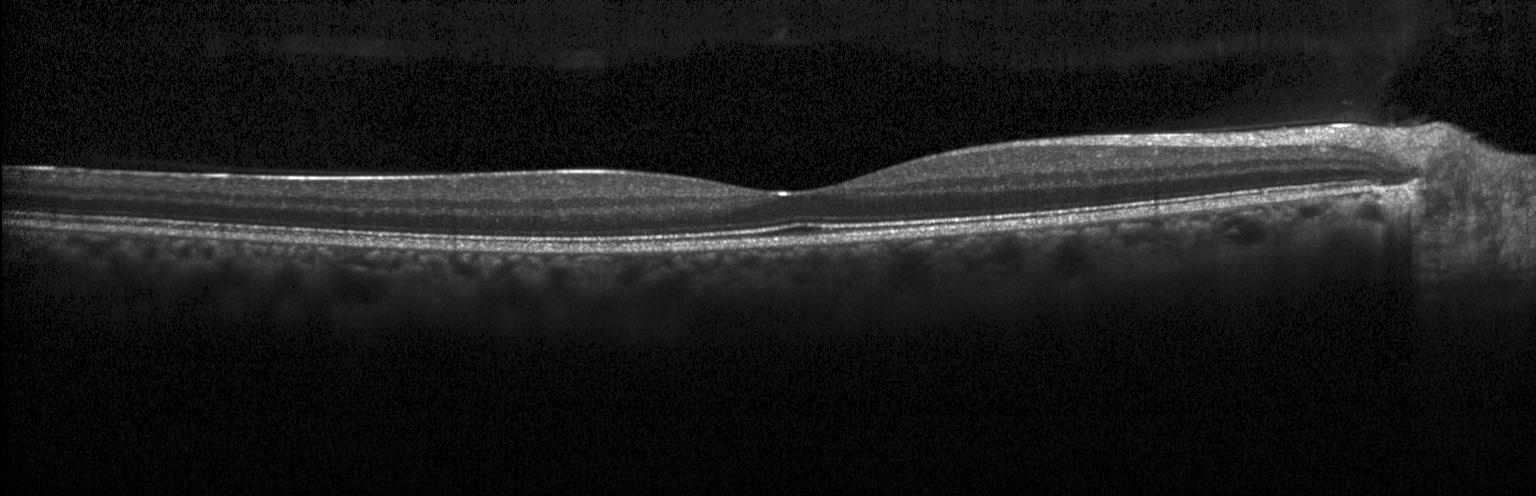
Finding: no choroidal neovascularization, no diabetic macular edema, and no drusen.